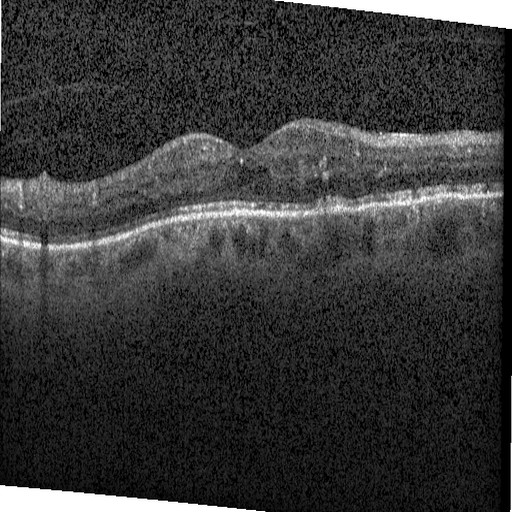 Retinal OCT cross-section; macular scan; SD-OCT.
Impression: diabetic macular edema (DME).